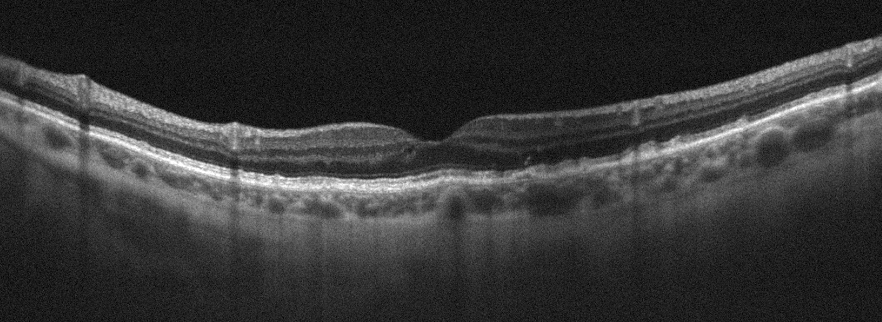

Right eye. OCT line scan.
Diagnosis: AMD.